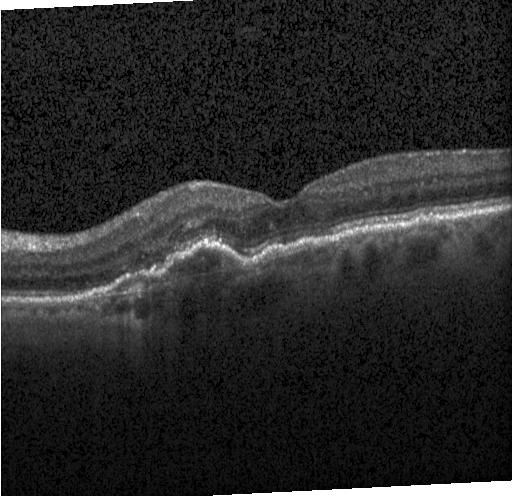 Heidelberg Spectralis OCT system, retinal OCT cross-section
Assessment: a choroidal neovascular membrane.